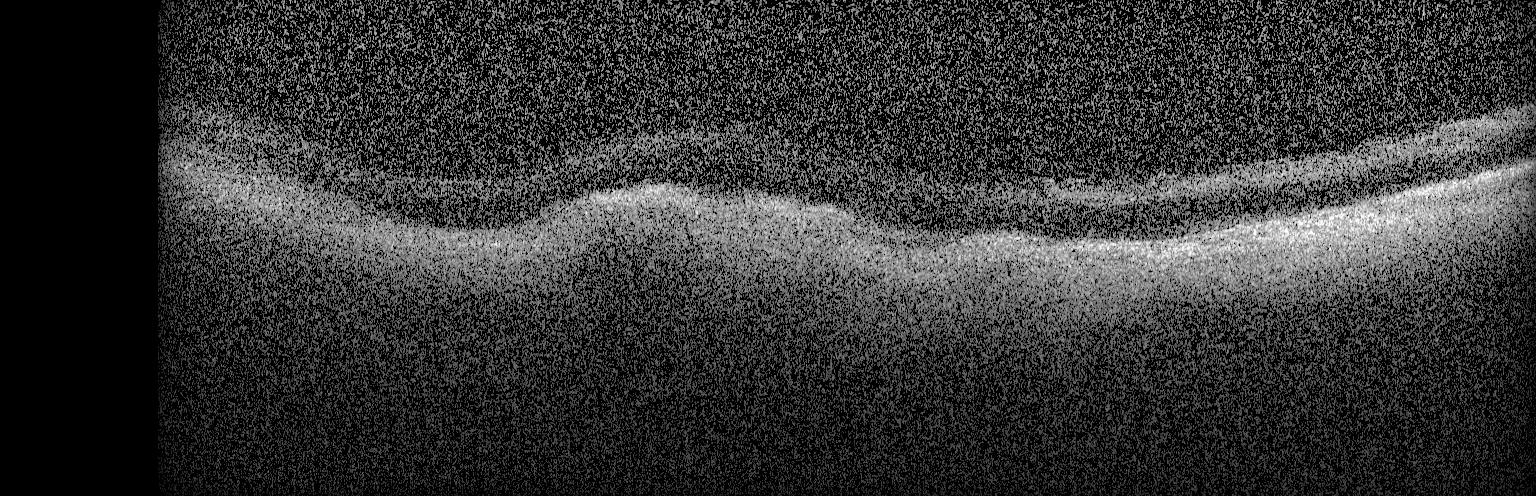
Macular OCT: a choroidal neovascular membrane.